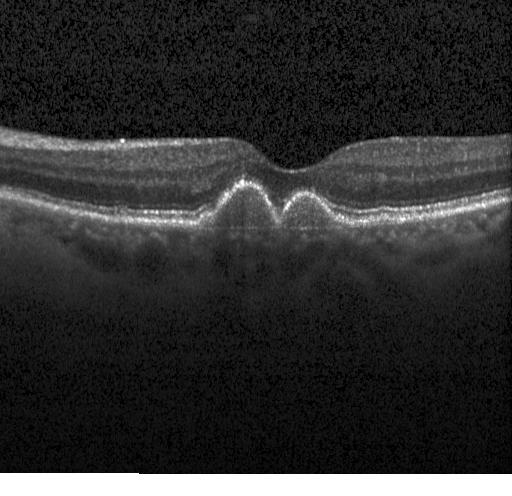 Optical coherence tomography scan. Horizontal scan through the fovea. Acquired on a Heidelberg Spectralis. SD-OCT.
Assessment: drusen.